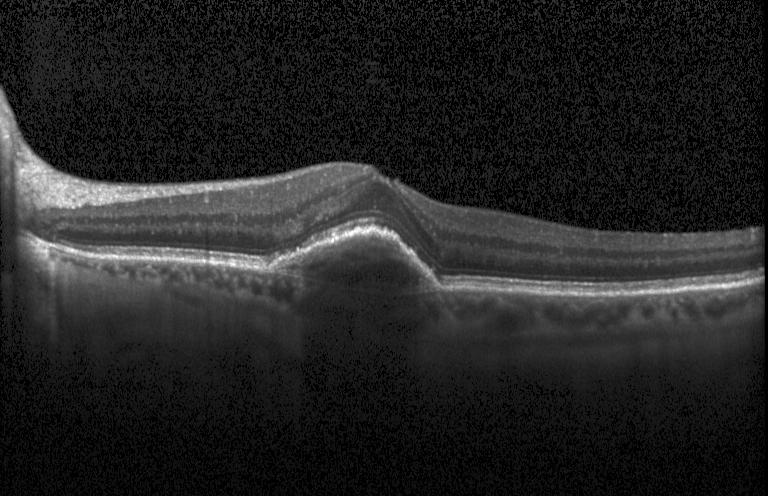

OCT B-scan showing a choroidal neovascular membrane.